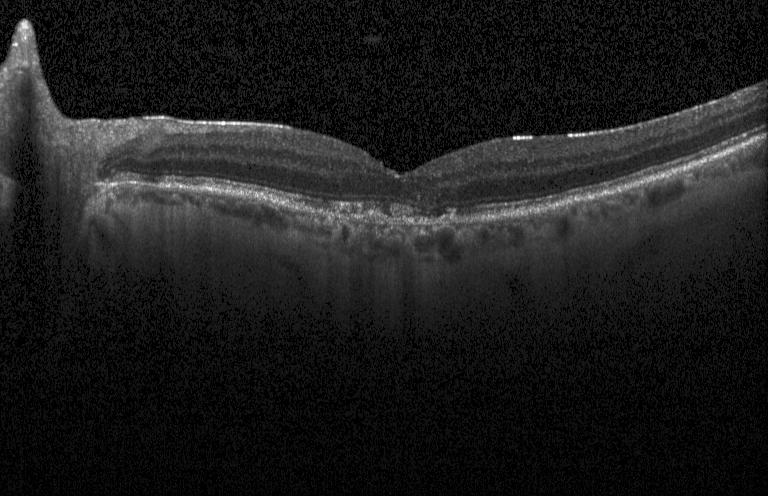

OCT B-scan showing a choroidal neovascular membrane.